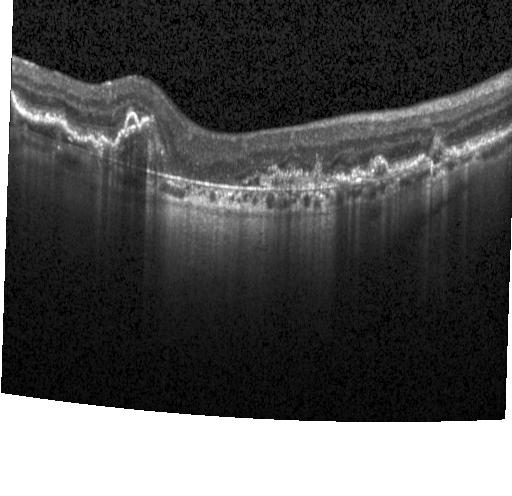
Impression: choroidal neovascularization.